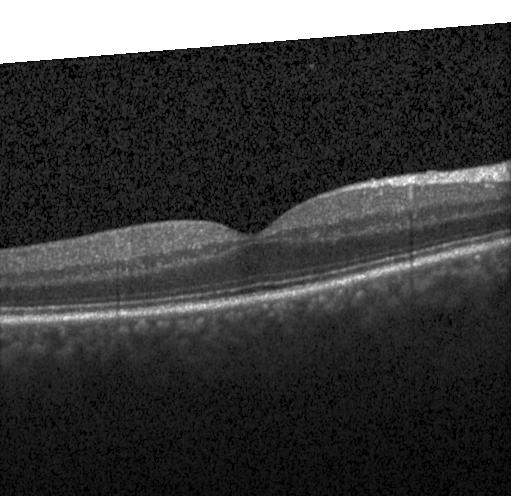
Diagnosis: no choroidal neovascularization, no diabetic macular edema, and no drusen.